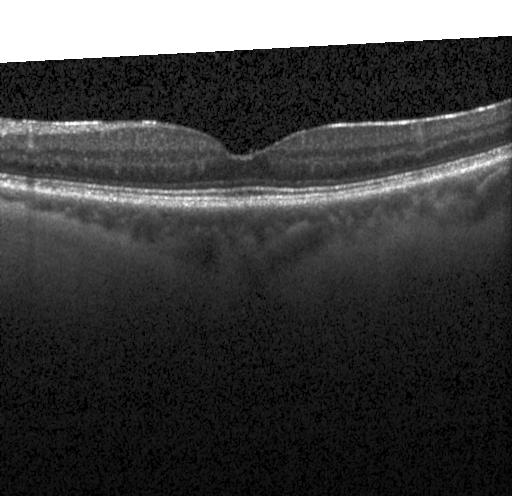

Dx: neither choroidal neovascularization, diabetic macular edema, nor drusen.